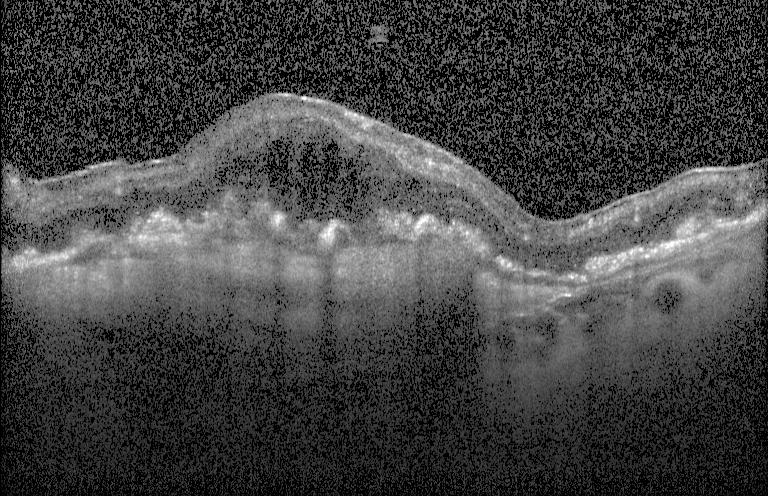

Retinal OCT B-scan, Heidelberg Spectralis, SD-OCT. Finding: a choroidal neovascular membrane.